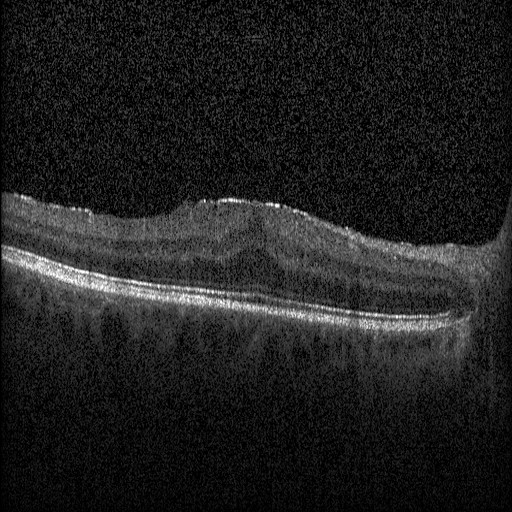
Horizontal scan through the fovea; SD-OCT; OCT B-scan; instrument: Heidelberg Spectralis
The scan shows DME.